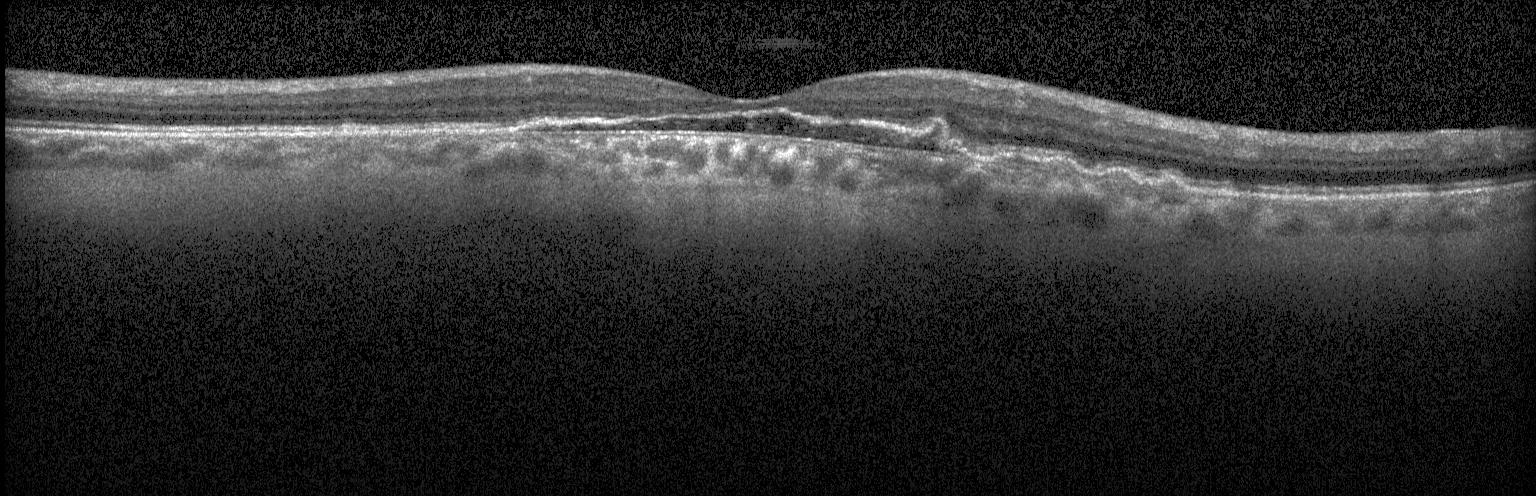

Retinal OCT B-scan, Heidelberg Spectralis. Impression: choroidal neovascularization (CNV).